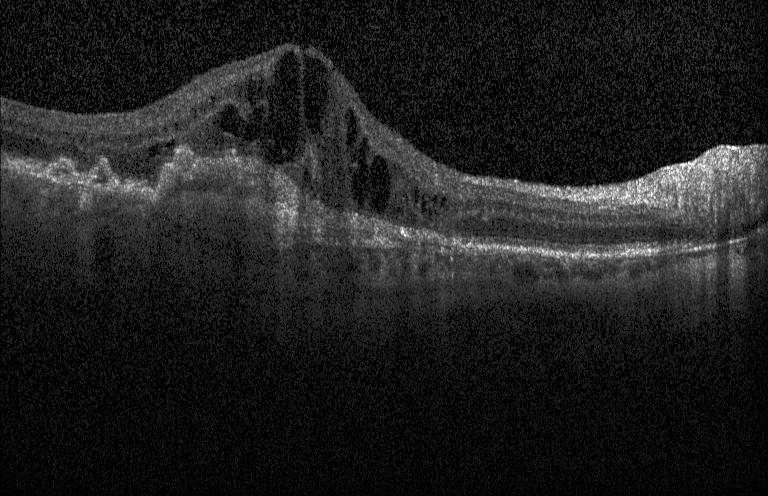 Heidelberg Spectralis OCT system; fovea-centered; retinal OCT B-scan; spectral-domain OCT
Diagnosis: a choroidal neovascular membrane.